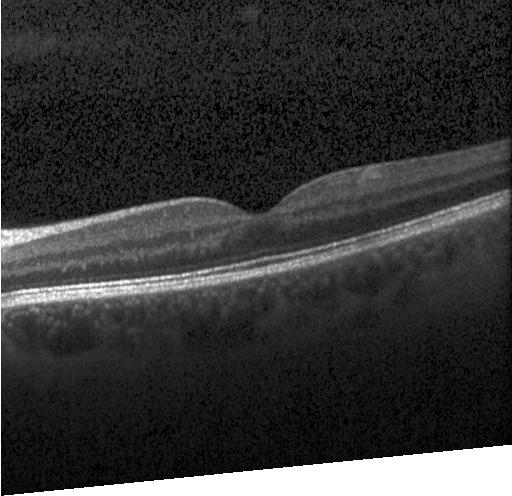 Retinal OCT B-scan.
Impression: no evidence of CNV, DME, or drusen.